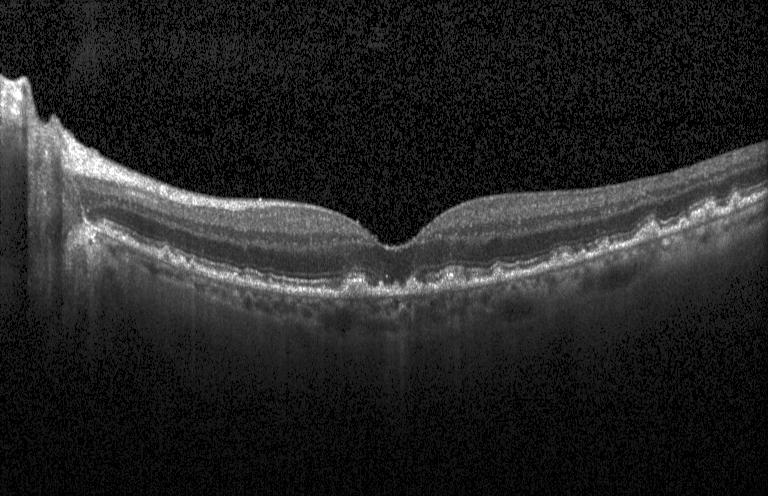
OCT B-scan · spectral-domain OCT
OCT finding: sub-RPE drusenoid deposits.